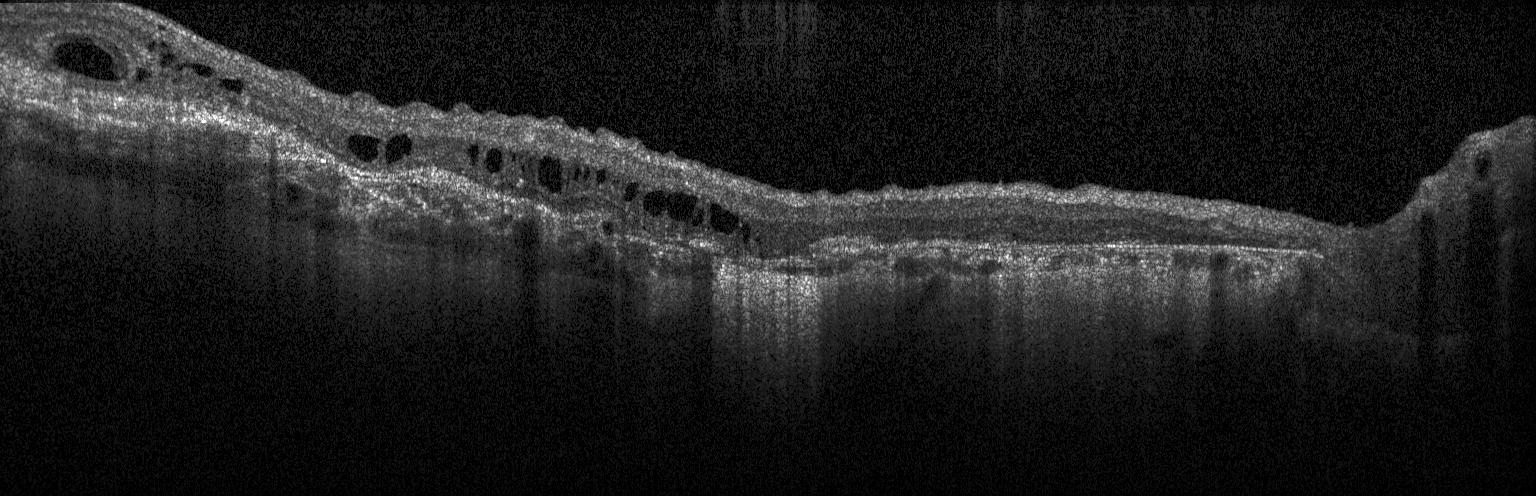
OCT finding: CNV.